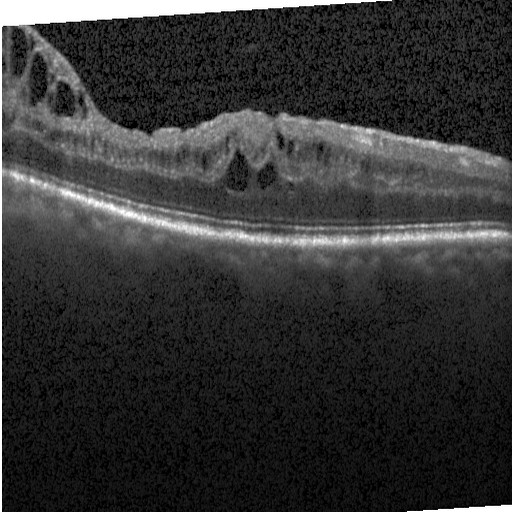

Fovea-centered; Heidelberg Spectralis OCT system; retinal OCT B-scan — Finding: diabetic macular edema (DME).